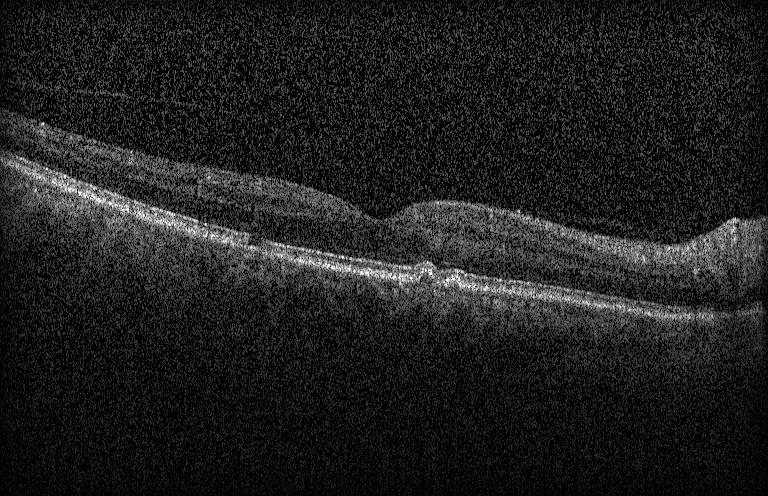 Retinal OCT cross-section showing drusen.